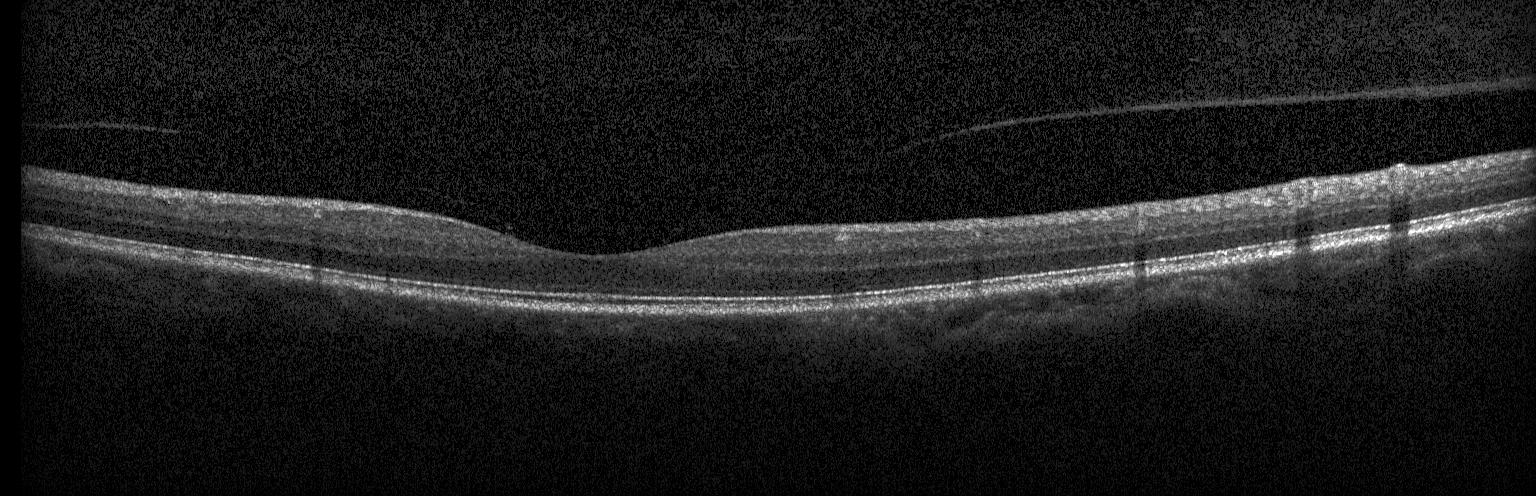 Heidelberg Spectralis, spectral-domain optical coherence tomography, optical coherence tomography B-scan
Diagnosis: neither choroidal neovascularization, diabetic macular edema, nor drusen.